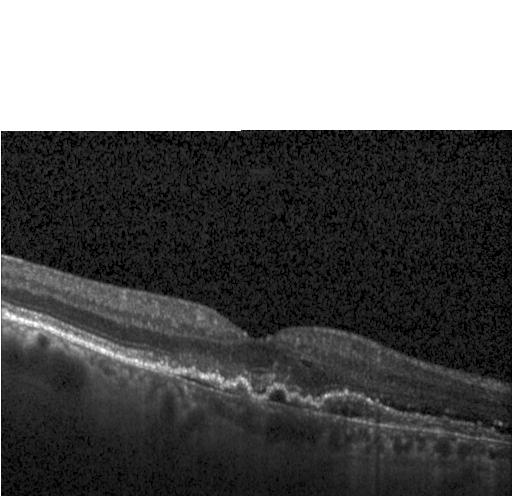
Instrument: Heidelberg Spectralis, retinal OCT cross-section — Assessment: choroidal neovascularization (CNV).